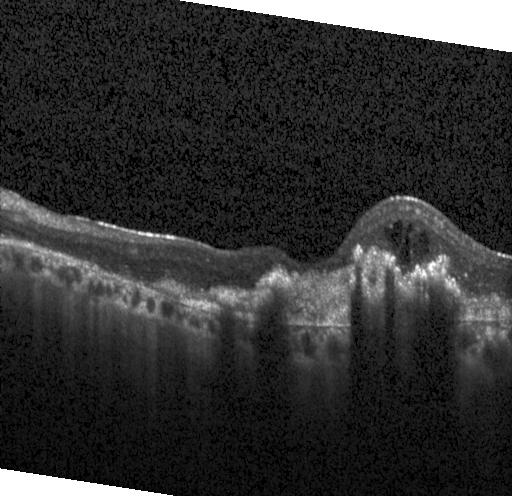

Retinal OCT B-scan, instrument: Heidelberg Spectralis, fovea-centered, spectral-domain optical coherence tomography. Finding: a choroidal neovascular membrane.